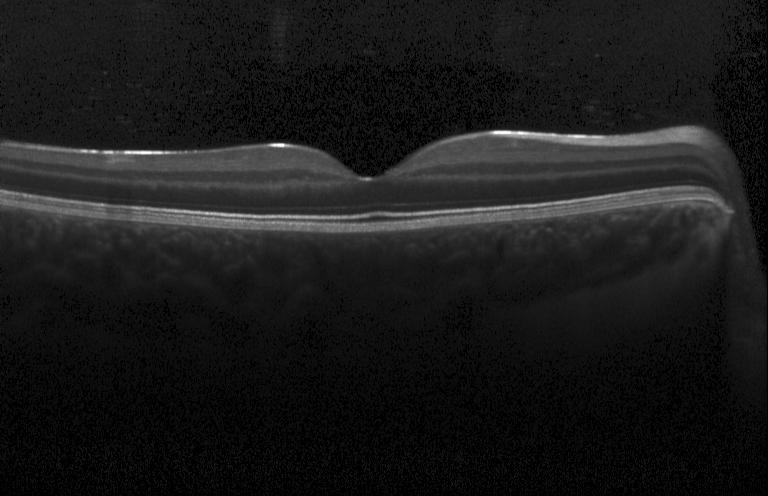
Retinal OCT B-scan. SD-OCT.
Impression: no CNV, no DME, and no drusen.